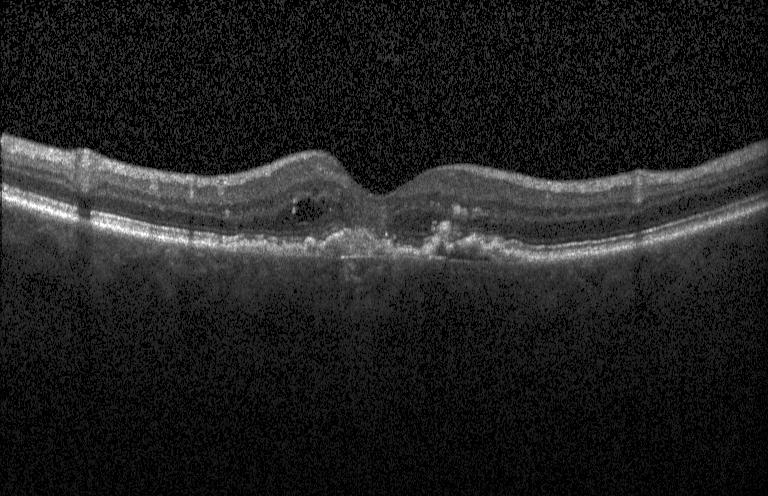
Assessment: a choroidal neovascular membrane.